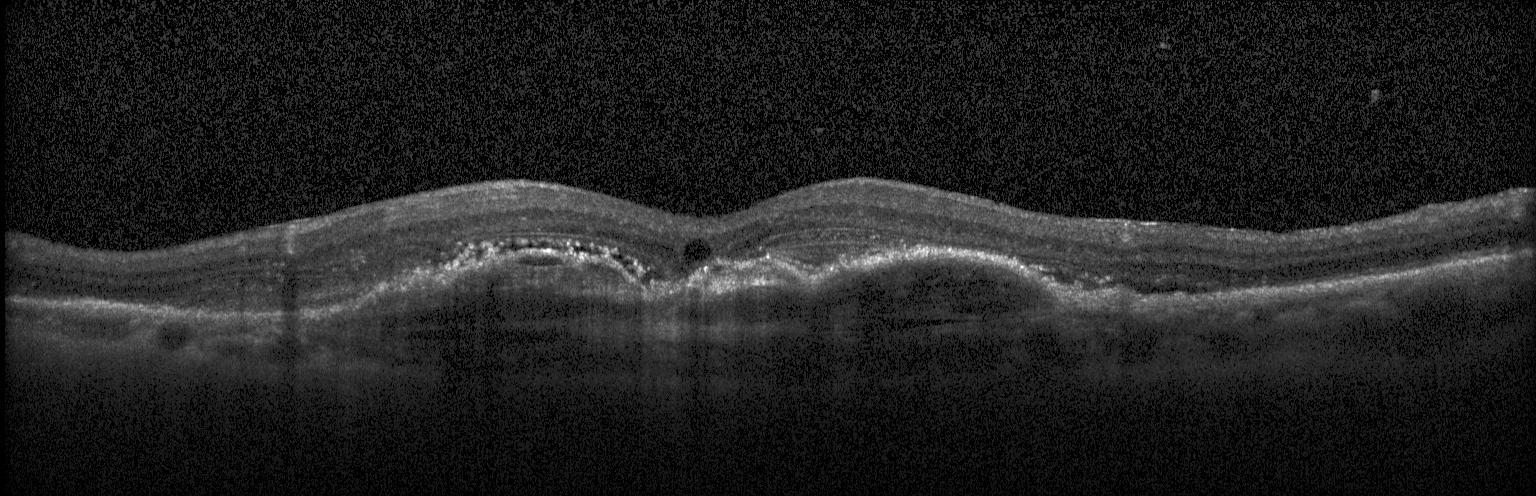
SD-OCT · optical coherence tomography scan · macular scan.
Impression: a choroidal neovascular membrane.